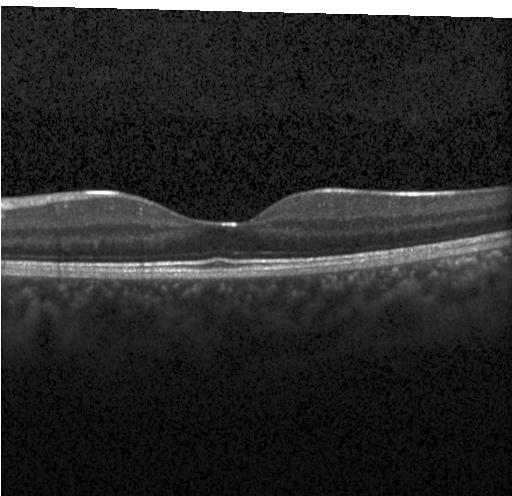
Retinal OCT cross-section
Impression: no choroidal neovascularization, diabetic macular edema, or drusen.